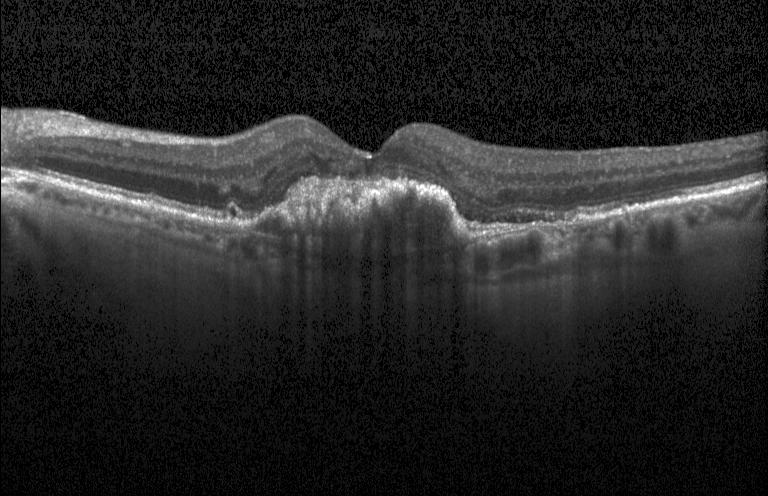 Acquired on a Heidelberg Spectralis, retinal OCT B-scan, spectral-domain OCT. Macular OCT: a choroidal neovascular membrane.